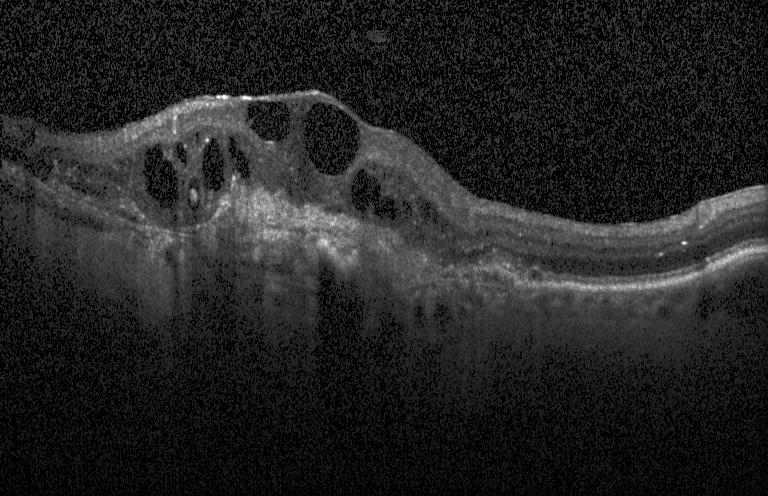 OCT scan showing a choroidal neovascular membrane.